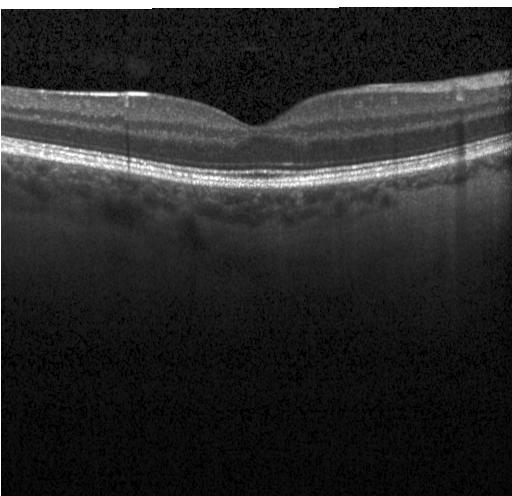

OCT finding: no CNV, DME, or drusen.